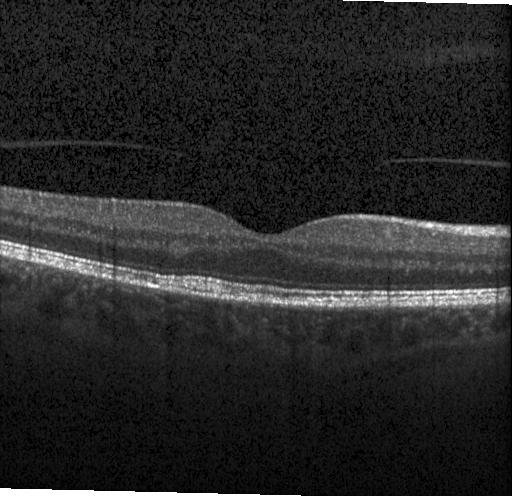
Finding: no choroidal neovascularization, diabetic macular edema, or drusen.